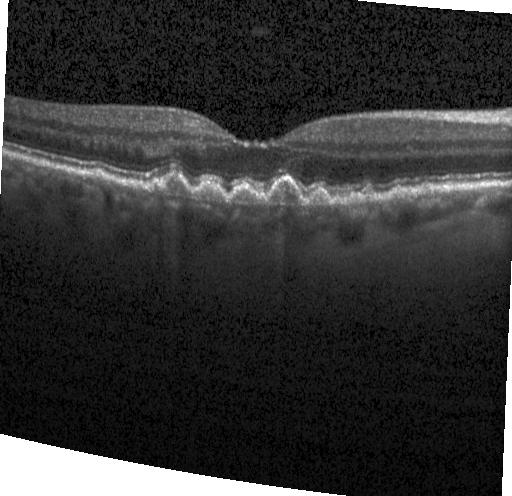 Macular OCT: multiple drusen.